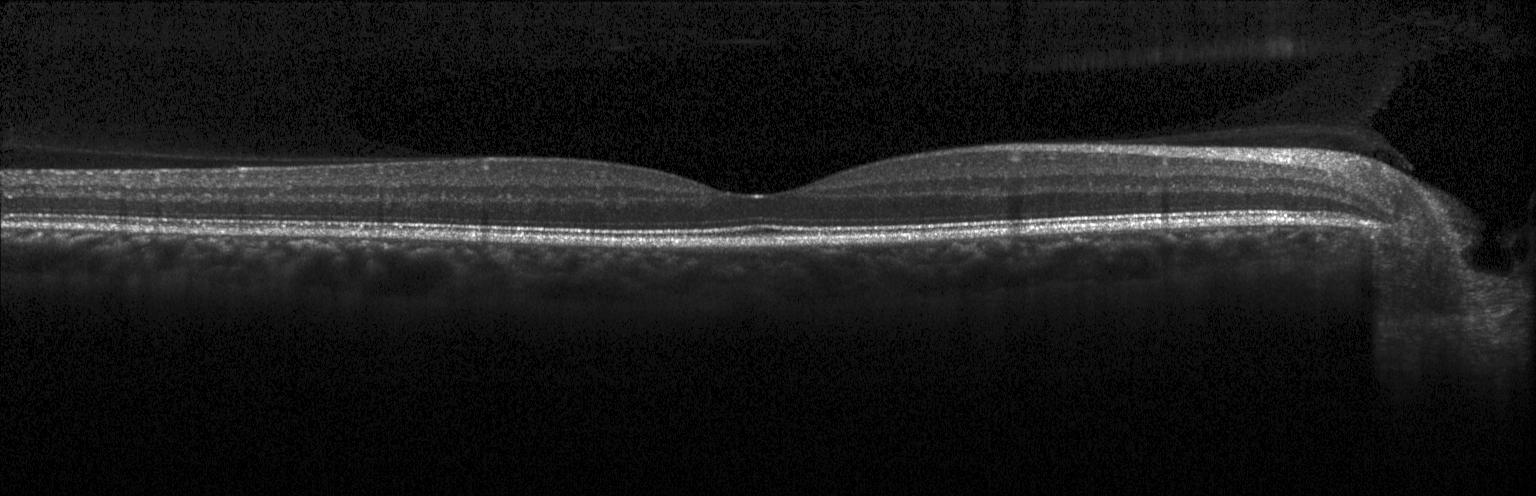

Horizontal scan through the fovea. Spectral-domain optical coherence tomography. Heidelberg Spectralis OCT system. Optical coherence tomography scan — Impression: no evidence of CNV, DME, or drusen.